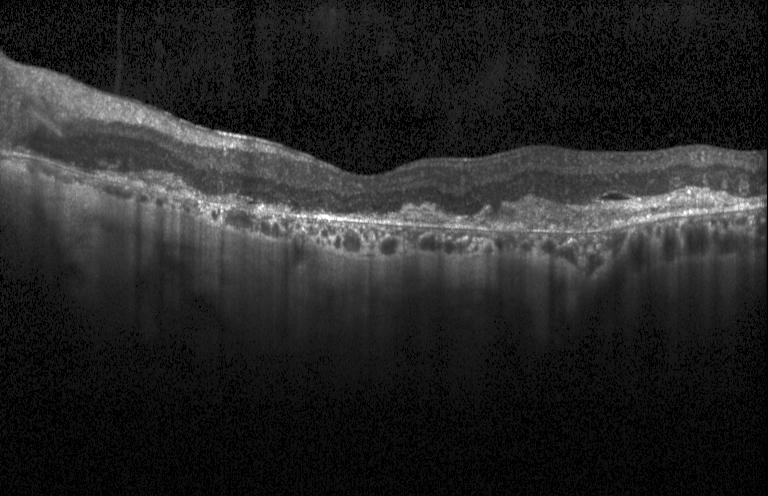

Acquired on a Heidelberg Spectralis. Spectral-domain optical coherence tomography. OCT line scan.
OCT finding: choroidal neovascularization.